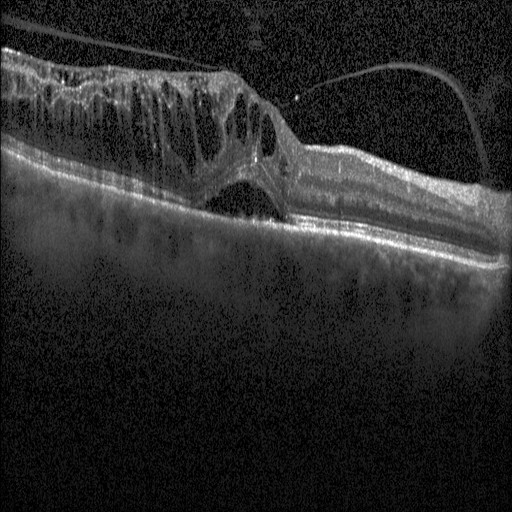 Retinal OCT cross-section; SD-OCT; acquired on a Heidelberg Spectralis
The scan shows DME.